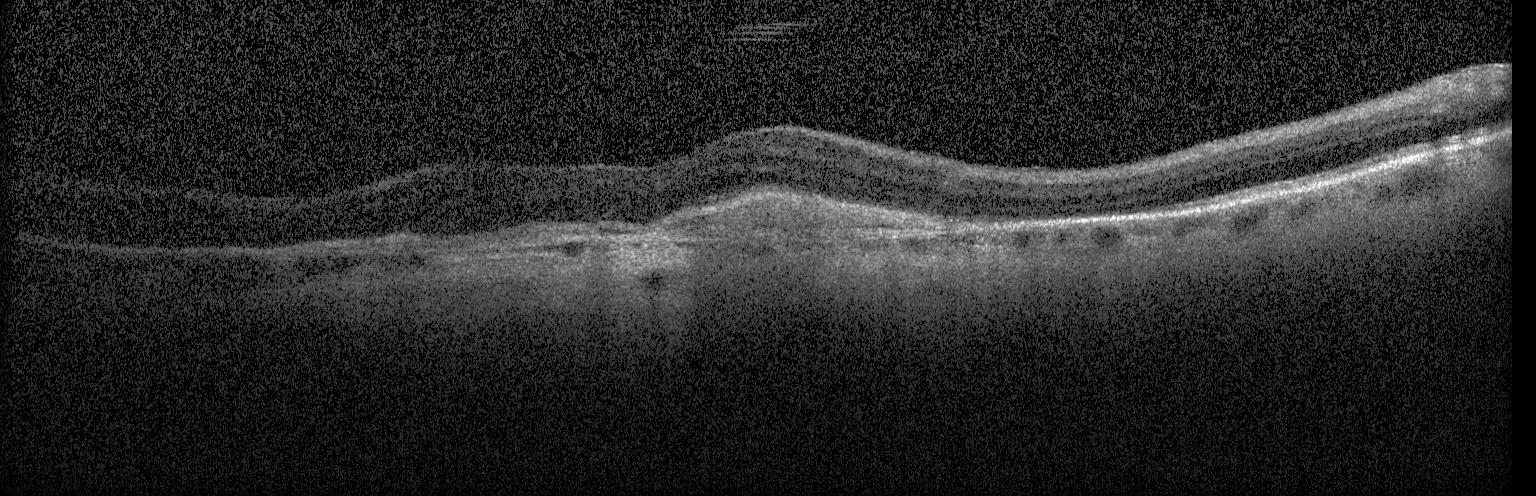
Optical coherence tomography B-scan
This B-scan demonstrates choroidal neovascularization.